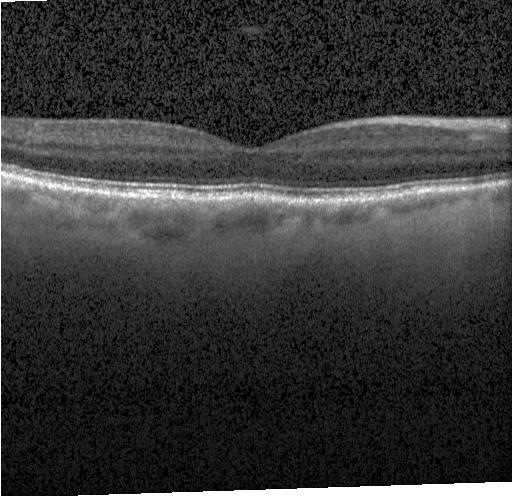

OCT scan showing no evidence of choroidal neovascularization, diabetic macular edema, or drusen.